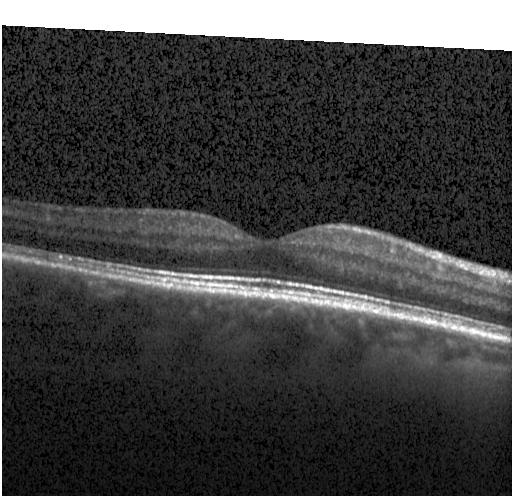
No evidence of CNV, DME, or drusen.